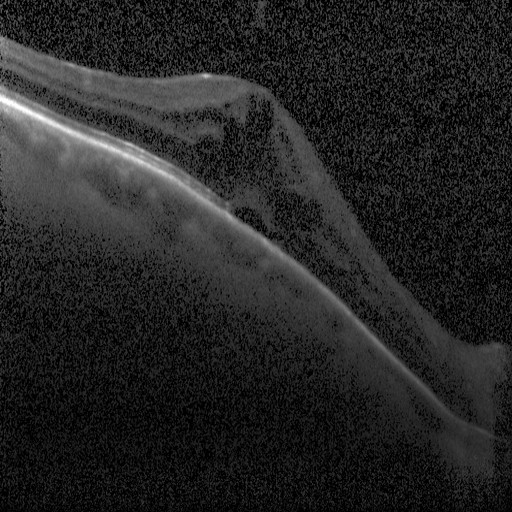
This B-scan demonstrates DME.